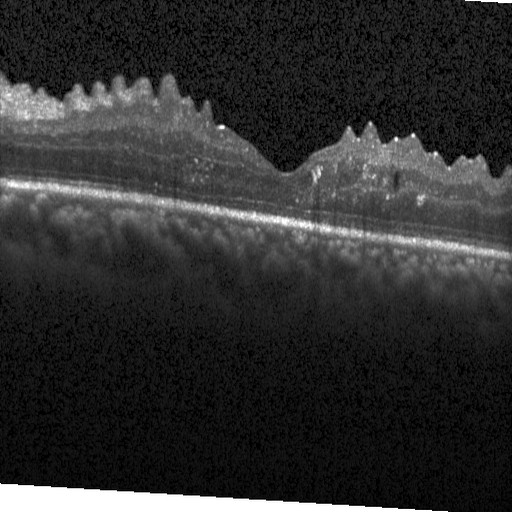 Impression: diabetic macular edema.